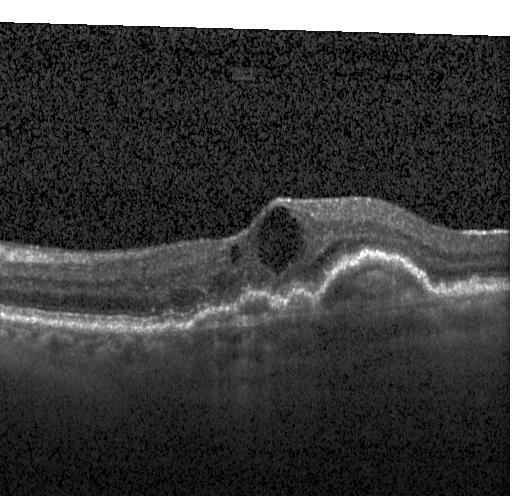

Instrument: Heidelberg Spectralis; retinal OCT cross-section.
OCT finding: a choroidal neovascular membrane.